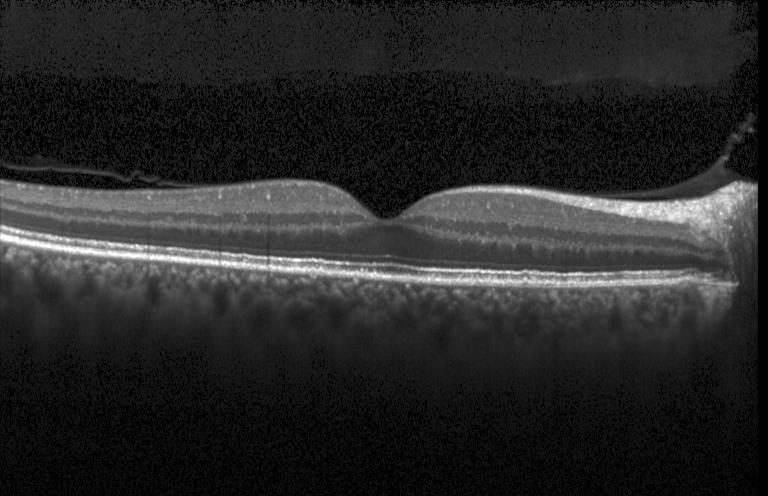
Horizontal scan through the fovea, instrument: Heidelberg Spectralis, retinal OCT cross-section. The scan shows neither CNV, DME, nor drusen.